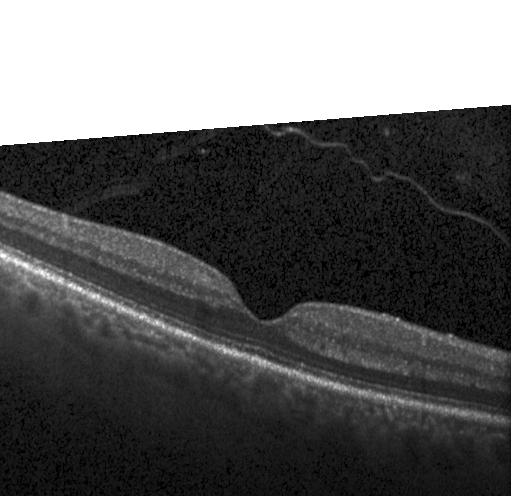 Optical coherence tomography scan. Assessment: no choroidal neovascularization, diabetic macular edema, or drusen.